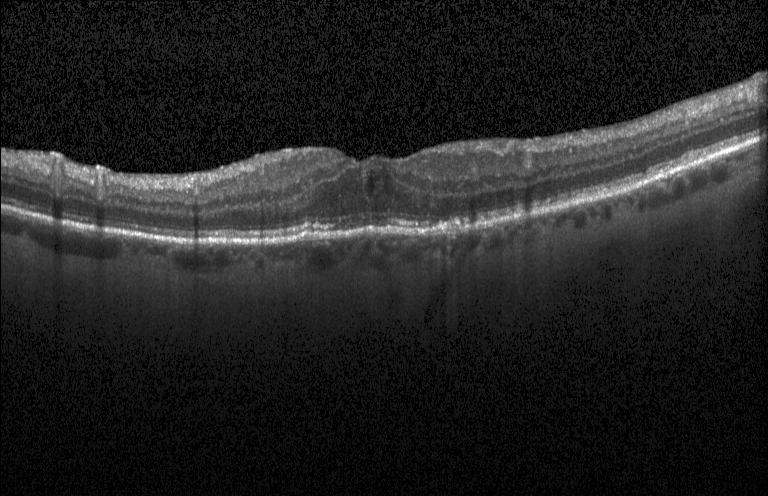 OCT finding: diabetic macular edema (DME).